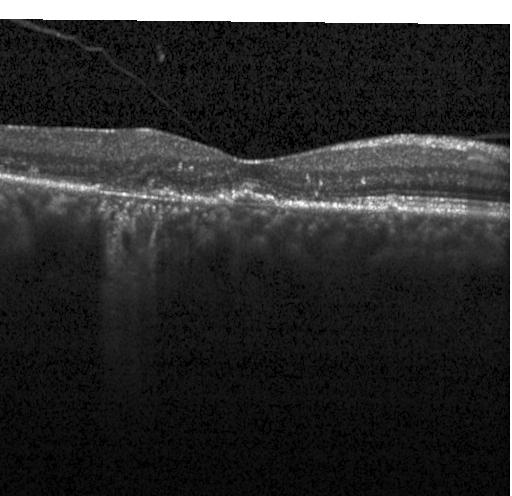 Optical coherence tomography scan · instrument: Heidelberg Spectralis · centered on the fovea. Macular OCT: a choroidal neovascular membrane.